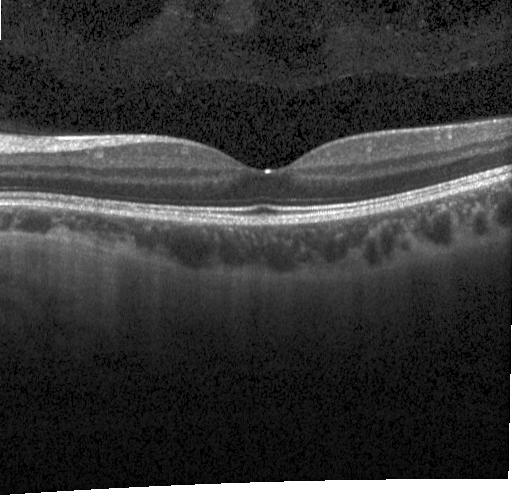
Impression: neither choroidal neovascularization, diabetic macular edema, nor drusen.